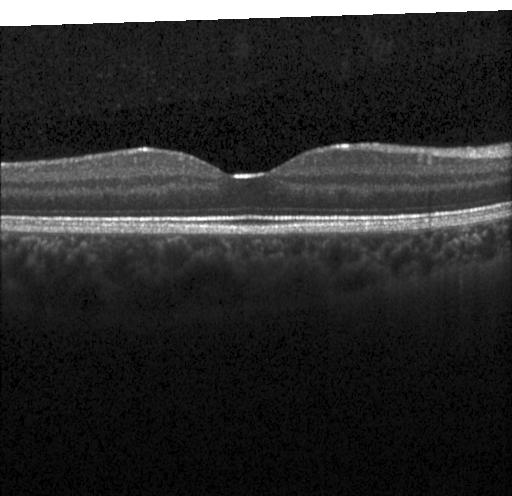 Retinal OCT cross-section · SD-OCT. Macular OCT: neither choroidal neovascularization, diabetic macular edema, nor drusen.